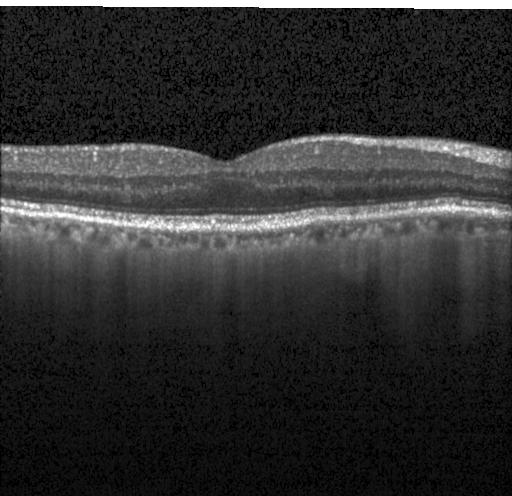 This B-scan demonstrates no CNV, DME, or drusen.